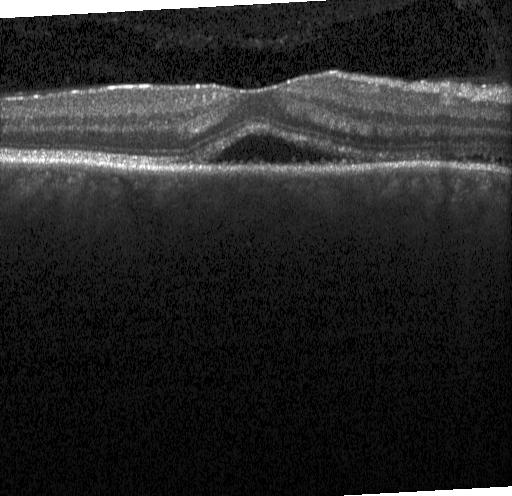

Optical coherence tomography B-scan — Impression: choroidal neovascularization.